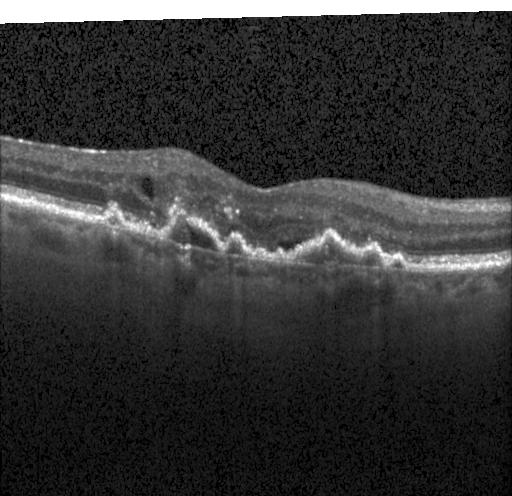

Impression: CNV.